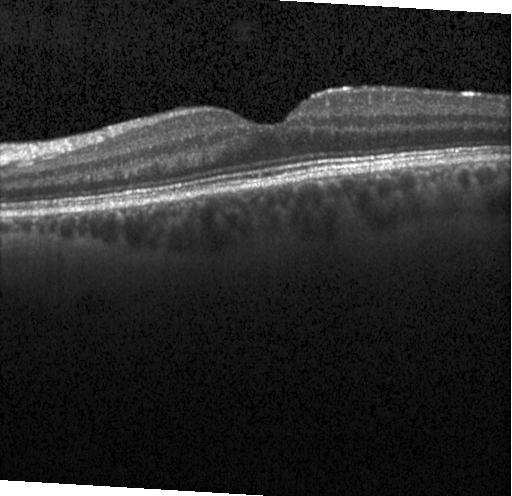

Optical coherence tomography B-scan. Heidelberg Spectralis. Horizontal scan through the fovea. Impression: no choroidal neovascularization, diabetic macular edema, or drusen.